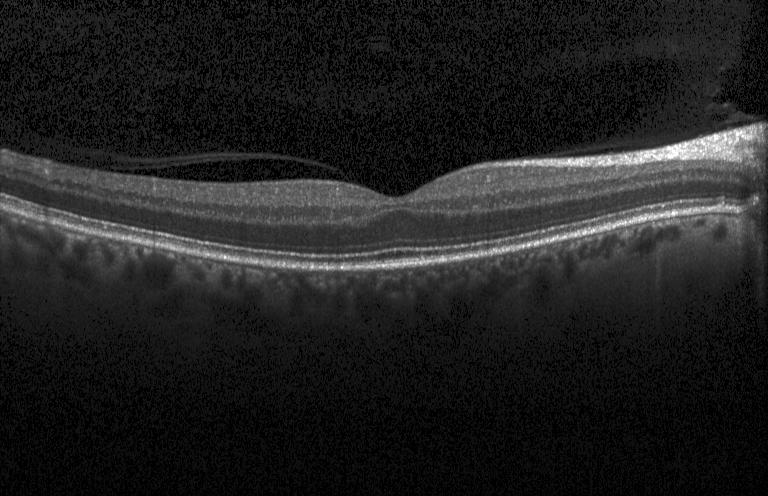 Retinal OCT cross-section, SD-OCT
No CNV, no DME, and no drusen.